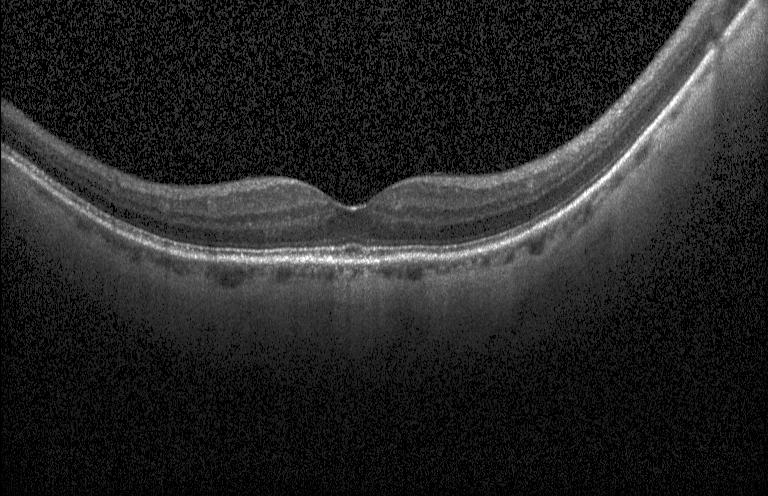
Through the macula · optical coherence tomography scan — Finding: no CNV, no DME, and no drusen.